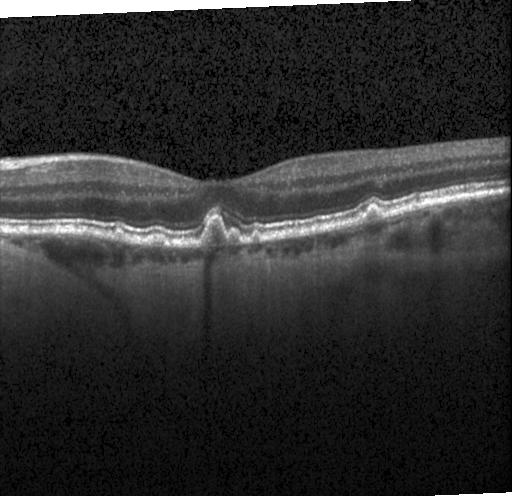

Retinal OCT cross-section showing sub-RPE drusenoid deposits.